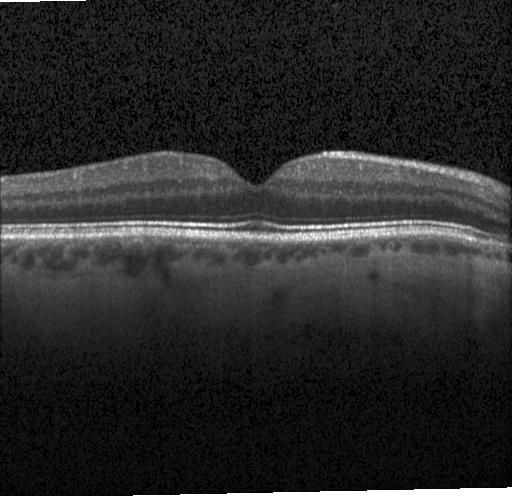
Optical coherence tomography B-scan; Heidelberg Spectralis OCT system
Impression: no evidence of choroidal neovascularization, diabetic macular edema, or drusen.